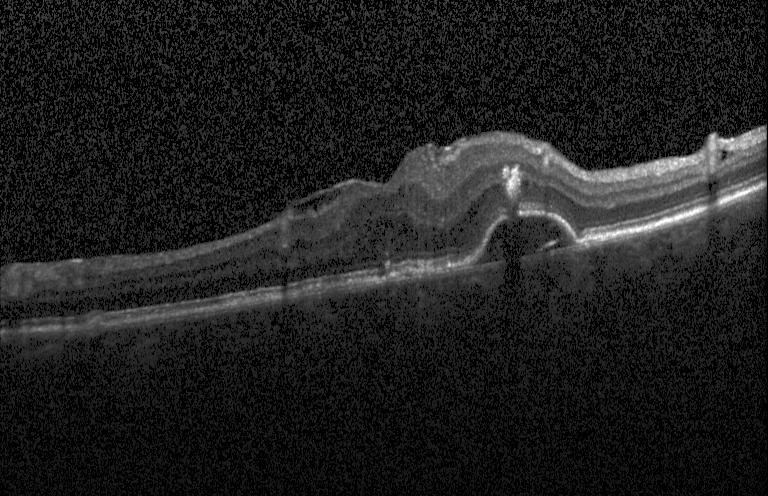 OCT finding: choroidal neovascularization (CNV).